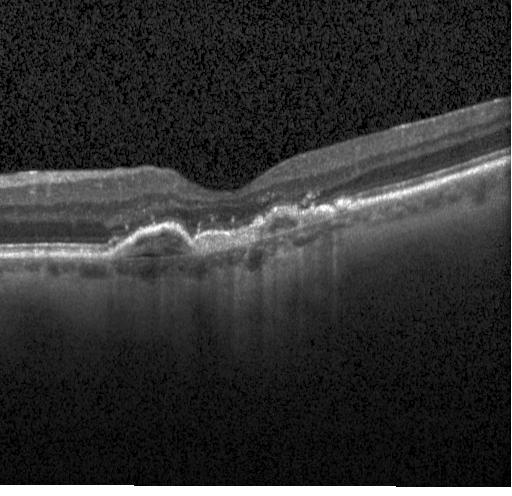

Horizontal scan through the fovea. Retinal OCT cross-section
Assessment: a choroidal neovascular membrane.